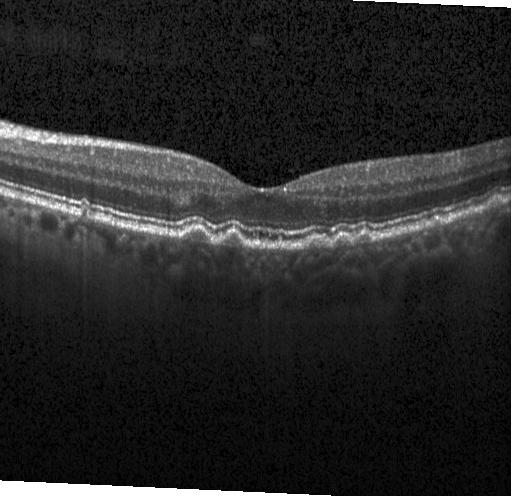 Centered on the fovea; OCT B-scan — Impression: drusen.